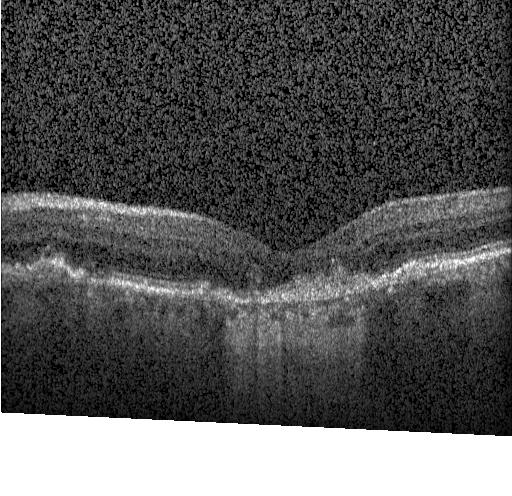
Retinal OCT cross-section · spectral-domain optical coherence tomography
Diagnosis: a choroidal neovascular membrane.